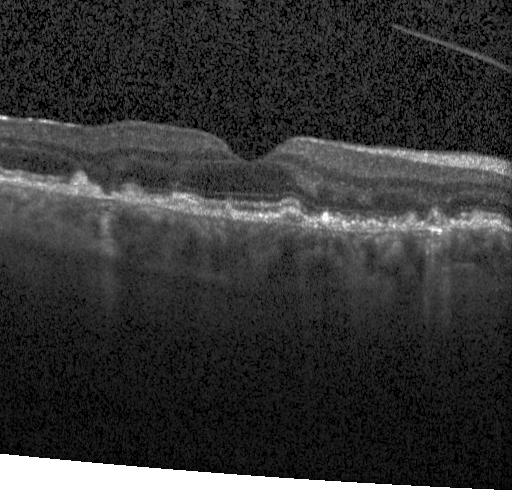
Impression: sub-RPE drusenoid deposits.